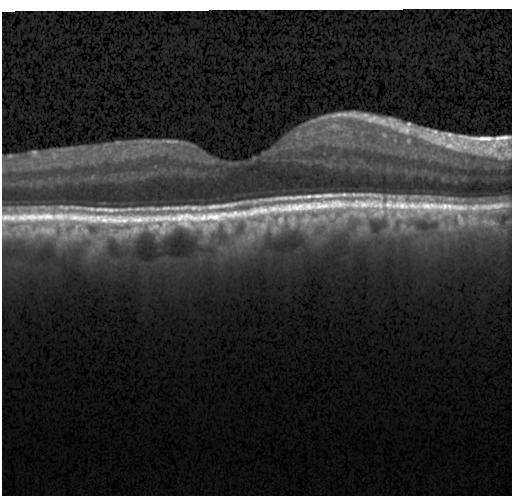 Optical coherence tomography B-scan.
Impression: no evidence of CNV, DME, or drusen.